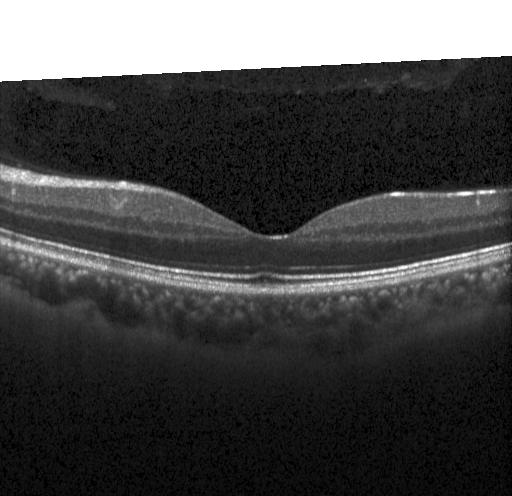

OCT scan showing no CNV, no DME, and no drusen.